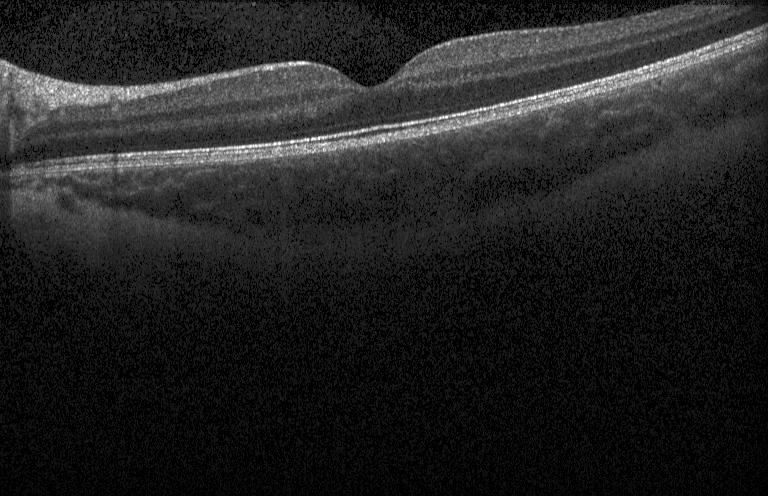

OCT line scan; instrument: Heidelberg Spectralis; macular scan; spectral-domain OCT.
No choroidal neovascularization, diabetic macular edema, or drusen.